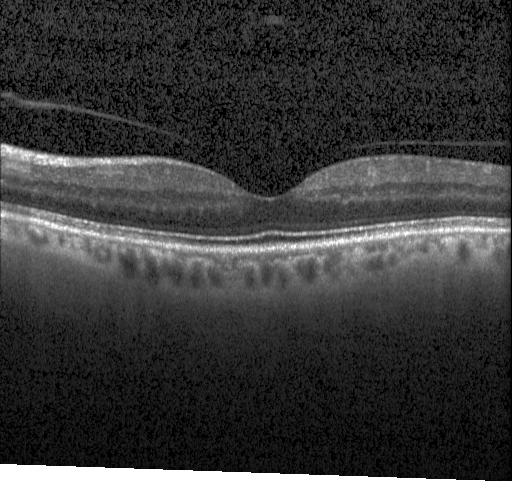 OCT B-scan showing no choroidal neovascularization, no diabetic macular edema, and no drusen.